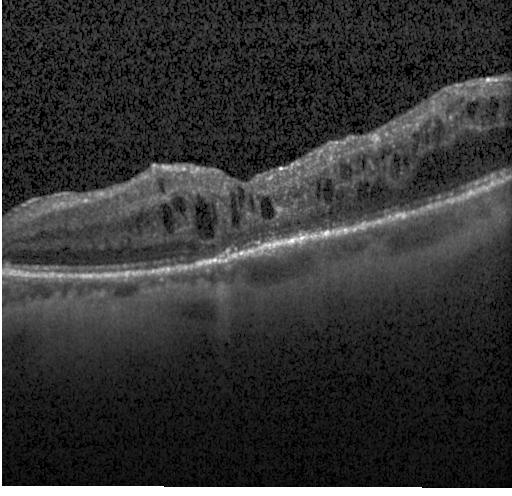
Heidelberg Spectralis; OCT line scan. Dx: diabetic macular edema (DME).